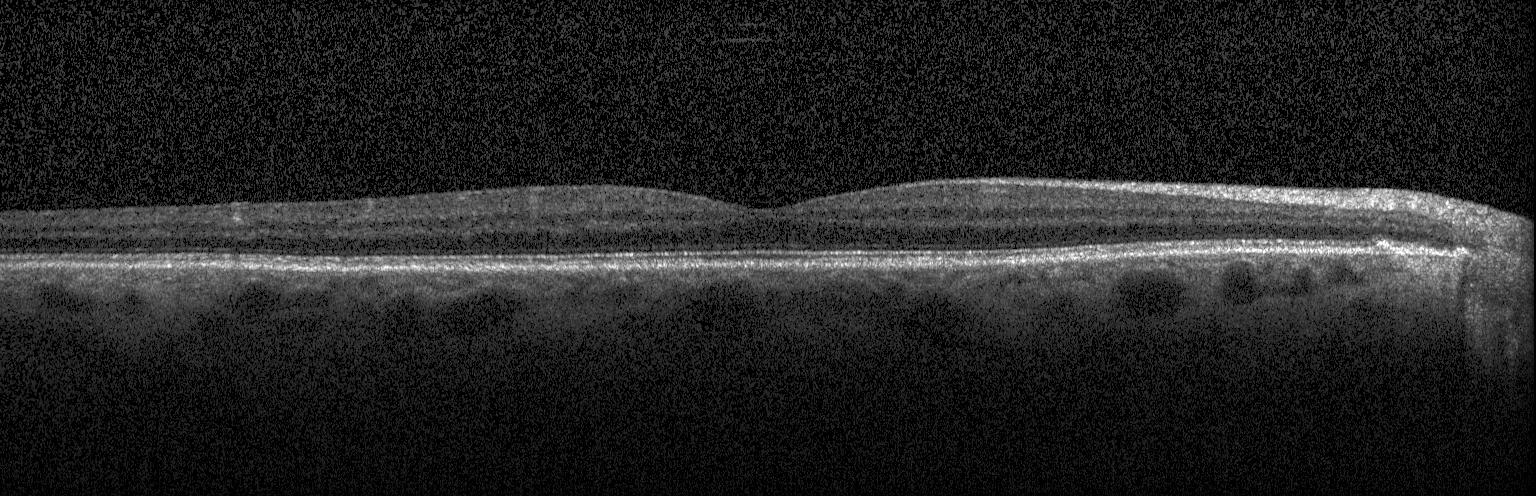

Optical coherence tomography scan · Heidelberg Spectralis · macular scan.
The scan shows no evidence of choroidal neovascularization, diabetic macular edema, or drusen.